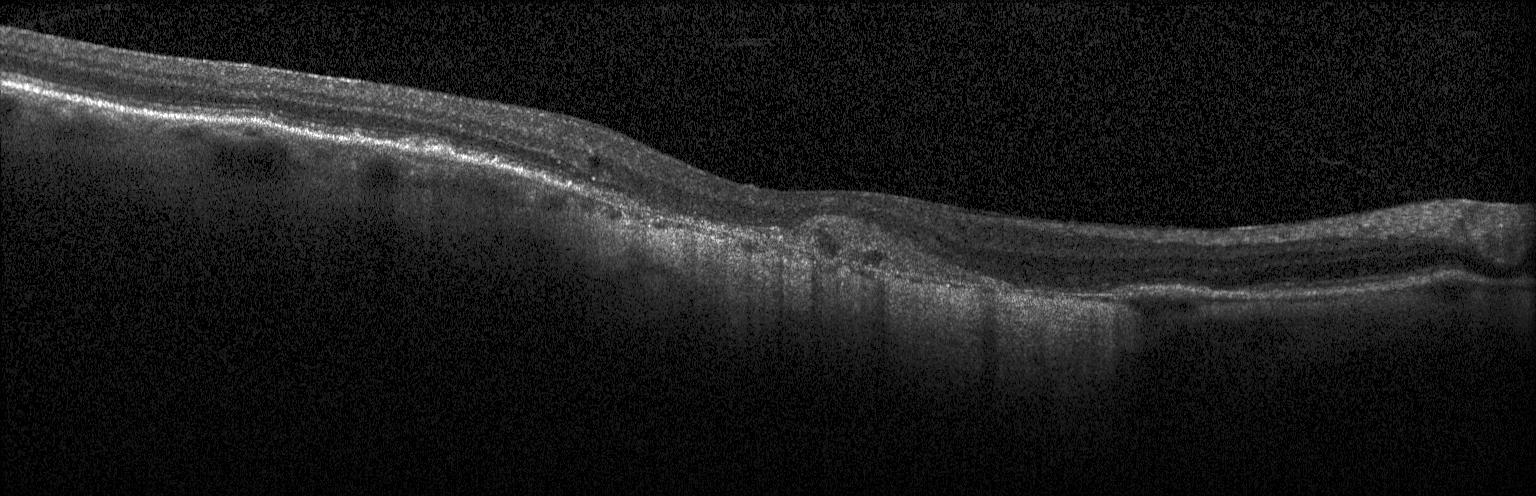
OCT B-scan, horizontal scan through the fovea — Assessment: a choroidal neovascular membrane.